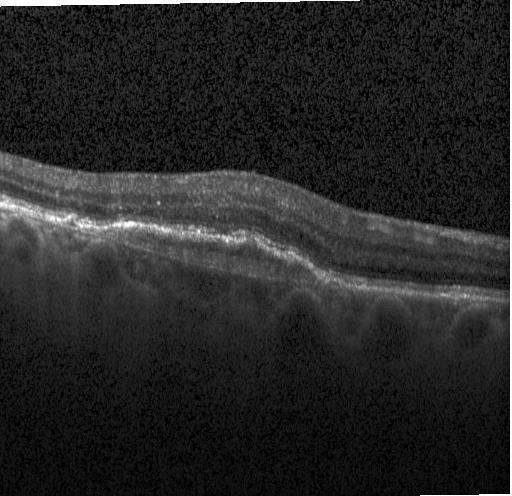
OCT B-scan — Macular OCT: choroidal neovascularization (CNV).